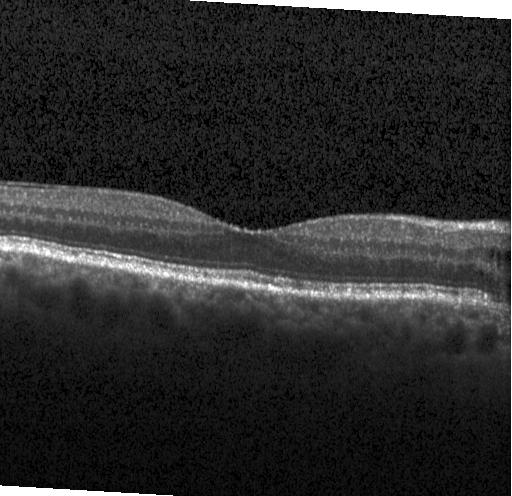
Macular OCT demonstrating diabetic macular edema (DME).